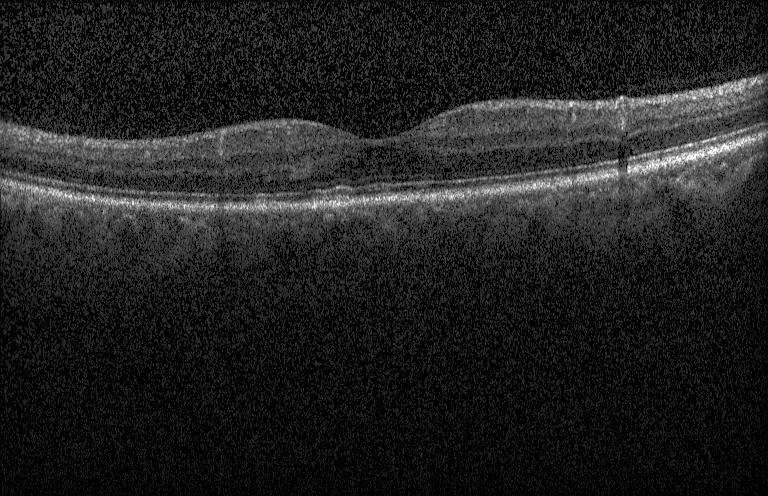
OCT scan showing no evidence of choroidal neovascularization, diabetic macular edema, or drusen.